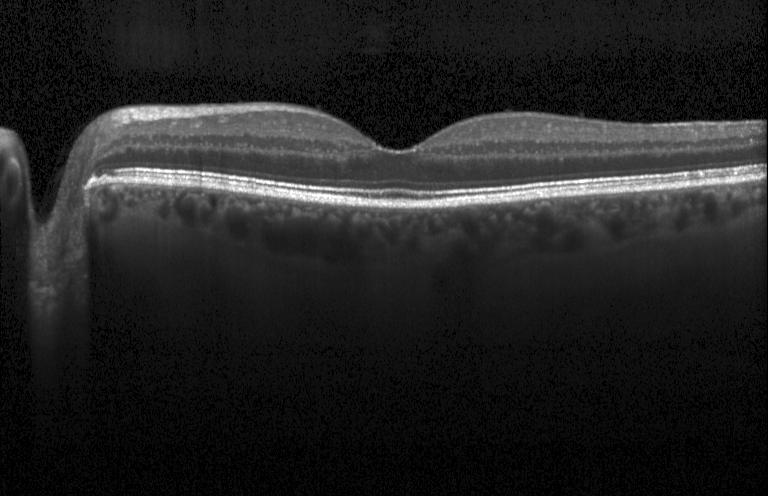 Impression: neither CNV, DME, nor drusen.